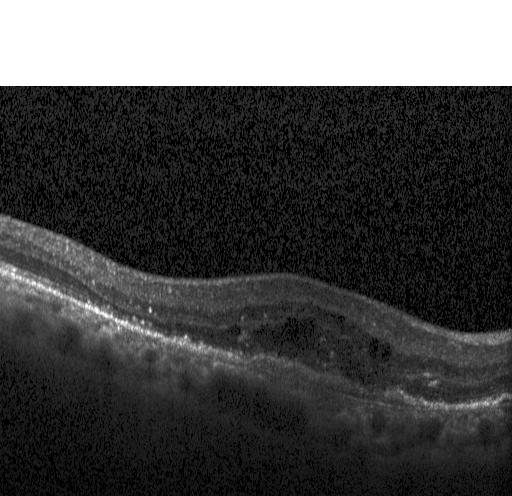
OCT finding: a choroidal neovascular membrane.